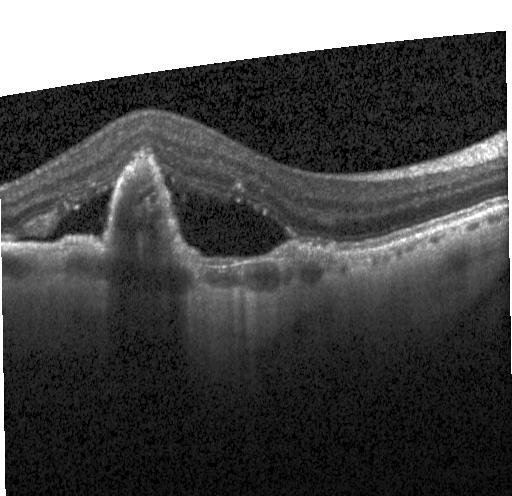
OCT line scan
Dx: choroidal neovascularization.